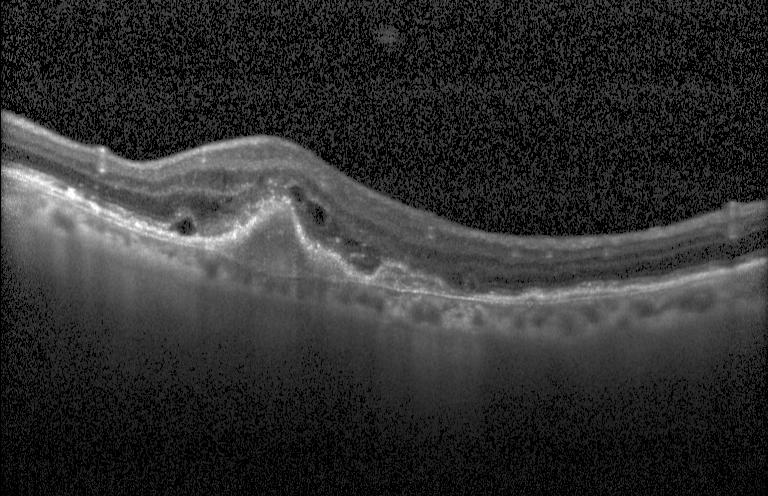 Impression: choroidal neovascularization (CNV).